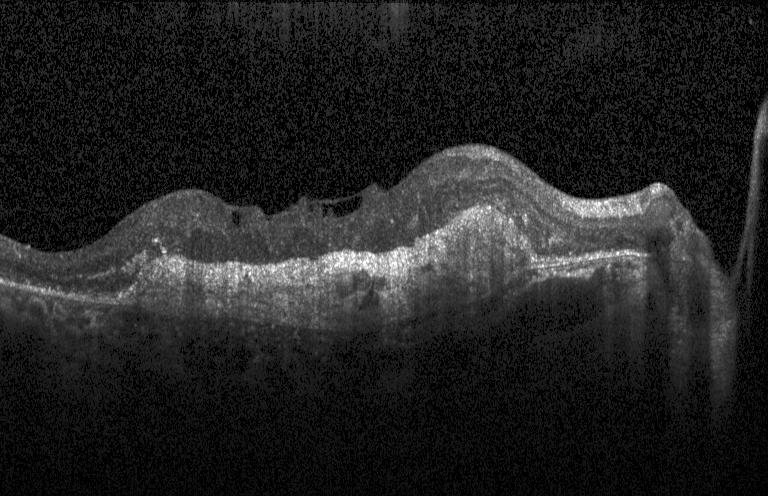 Acquired on a Heidelberg Spectralis; retinal OCT cross-section — Assessment: choroidal neovascularization.